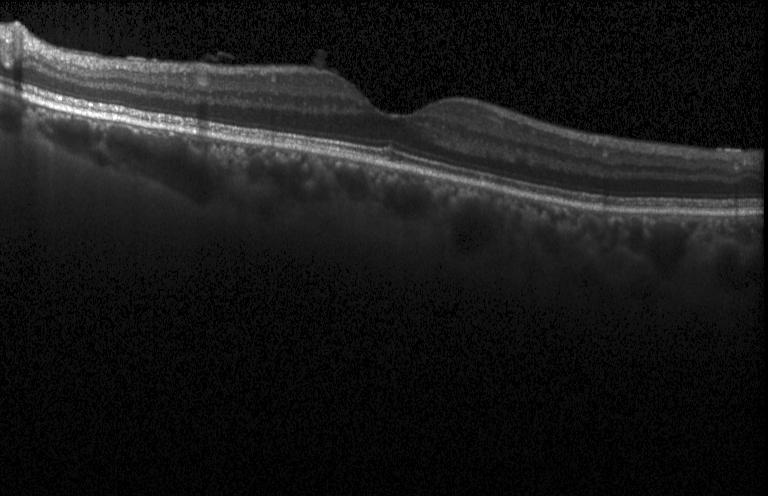

Retinal OCT B-scan. This B-scan demonstrates neither choroidal neovascularization, diabetic macular edema, nor drusen.